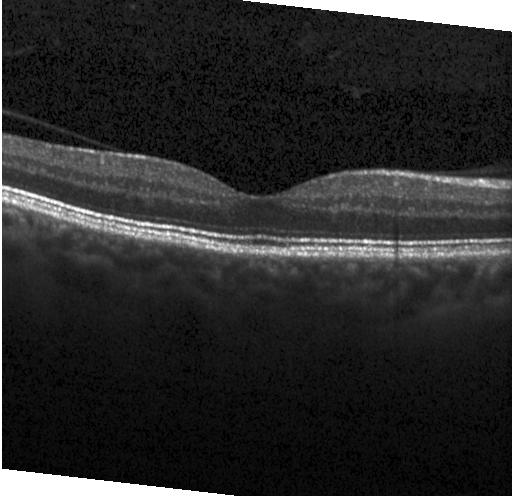
OCT line scan.
No choroidal neovascularization, no diabetic macular edema, and no drusen.